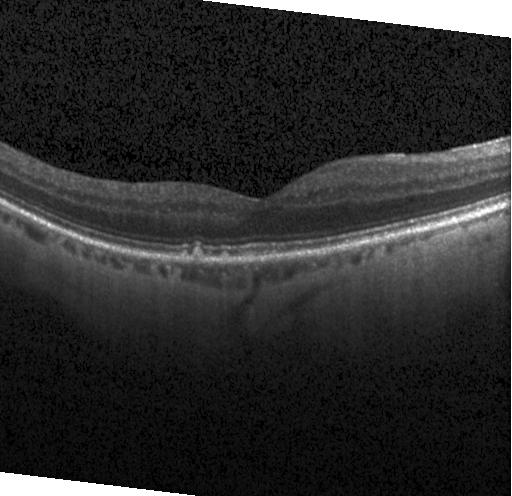
Retinal OCT B-scan. SD-OCT. Assessment: multiple drusen.